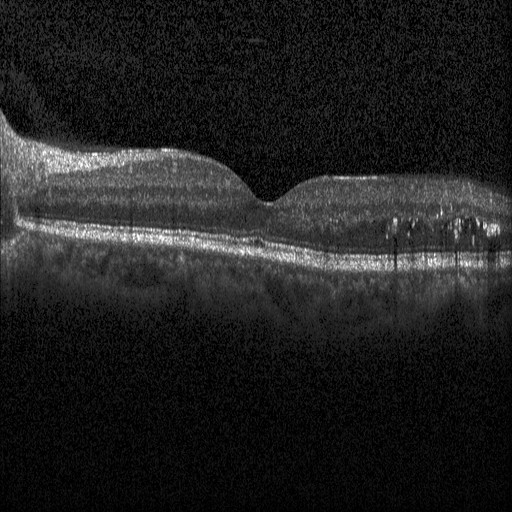
Spectral-domain OCT B-scan: diabetic macular edema (DME).